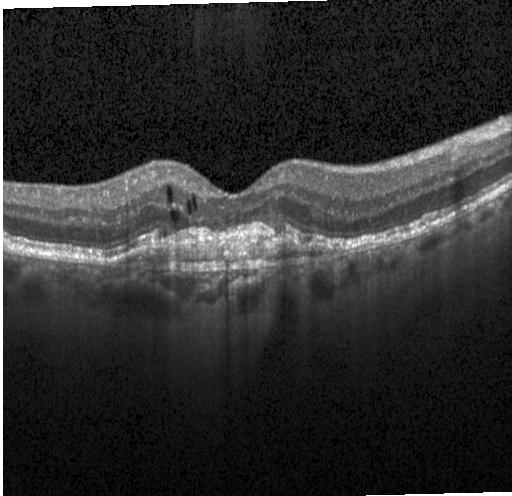 Spectral-domain optical coherence tomography. Retinal OCT B-scan. Impression: a choroidal neovascular membrane.